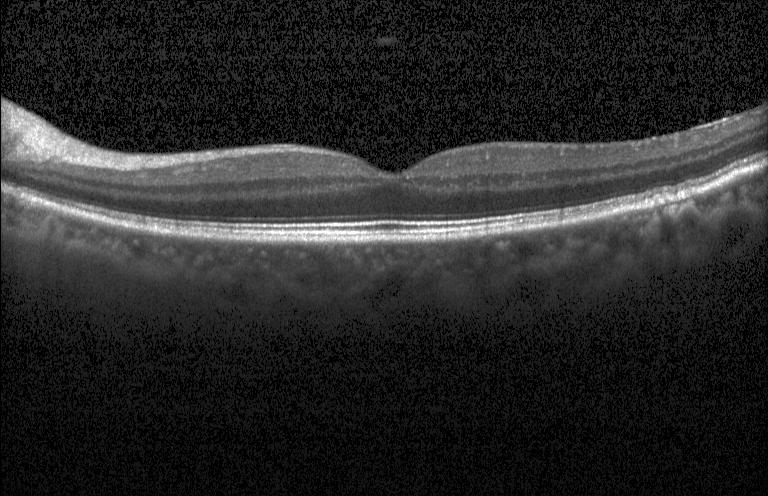

Spectral-domain OCT, retinal OCT cross-section — Diagnosis: no choroidal neovascularization, diabetic macular edema, or drusen.